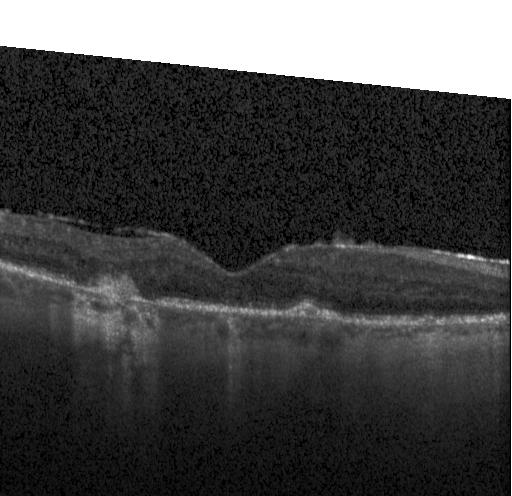

Optical coherence tomography B-scan · centered on the fovea.
Assessment: choroidal neovascularization (CNV).